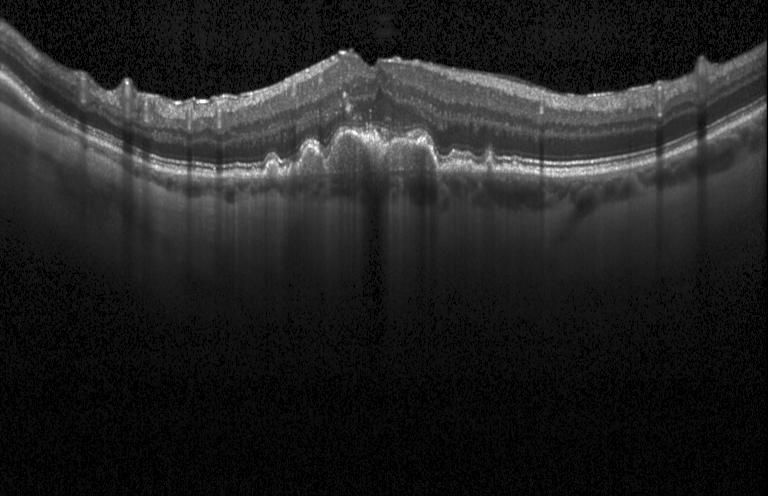

Heidelberg Spectralis OCT system, OCT line scan, spectral-domain optical coherence tomography.
OCT finding: sub-RPE drusenoid deposits.